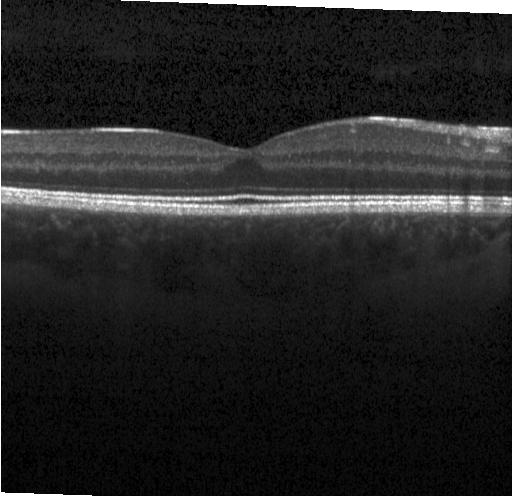
Heidelberg Spectralis OCT system · OCT B-scan · horizontal scan through the fovea.
Impression: no choroidal neovascularization, diabetic macular edema, or drusen.